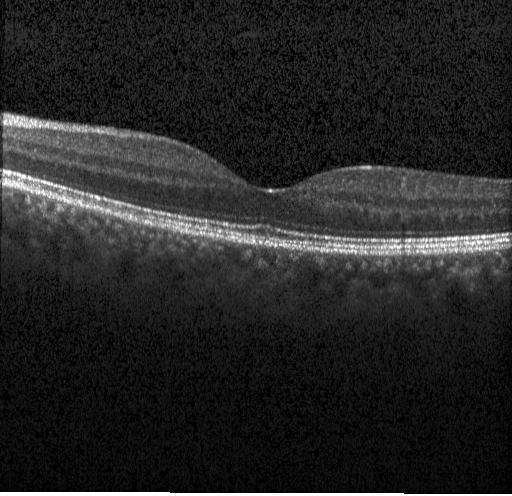 Retinal OCT cross-section, Heidelberg Spectralis OCT system.
OCT finding: no evidence of CNV, DME, or drusen.